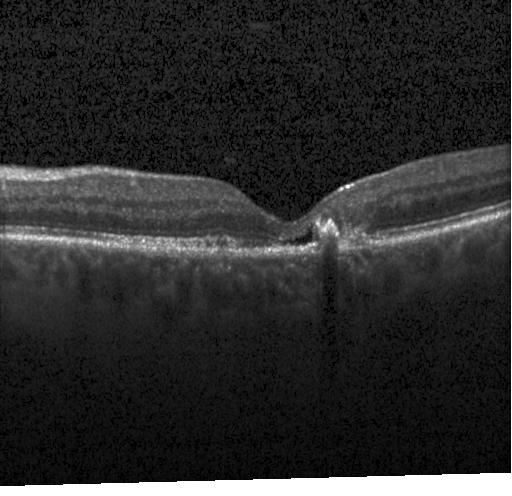 SD-OCT, optical coherence tomography scan.
A choroidal neovascular membrane.